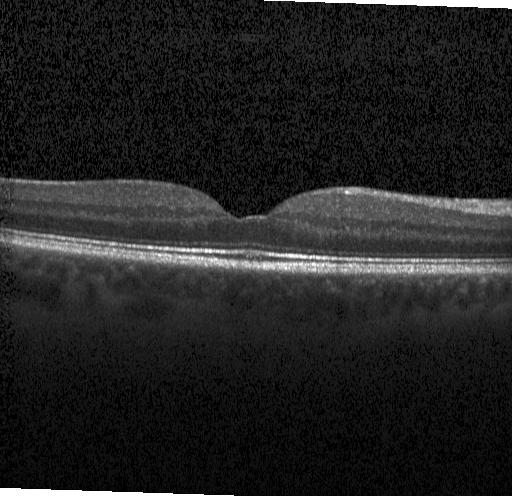
Heidelberg Spectralis; OCT line scan; fovea-centered; SD-OCT. Dx: no evidence of choroidal neovascularization, diabetic macular edema, or drusen.